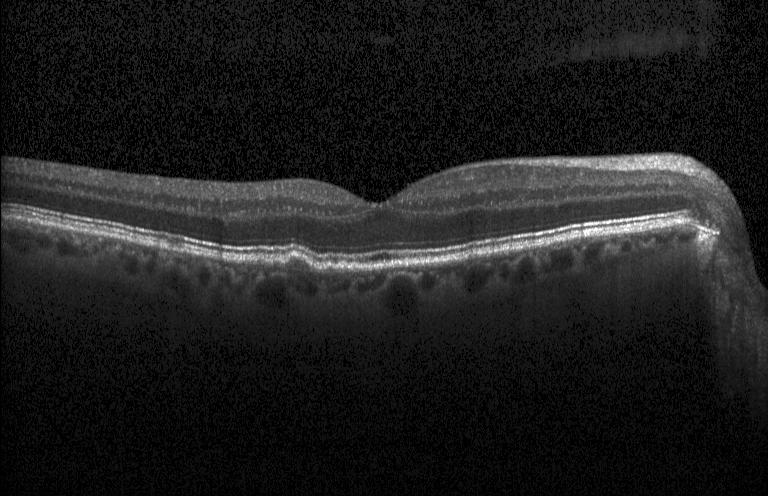

OCT B-scan; horizontal scan through the fovea; SD-OCT. Diagnosis: sub-RPE drusenoid deposits.